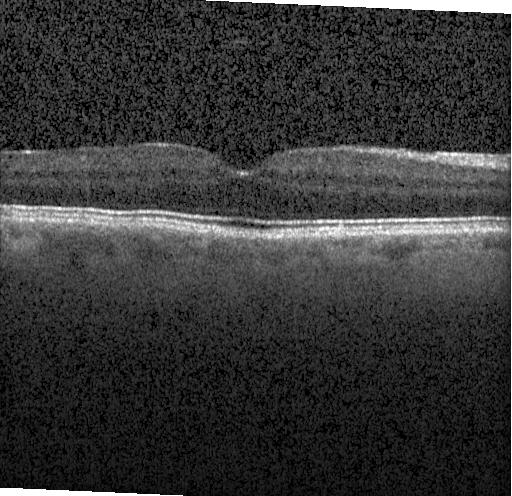

Spectral-domain OCT B-scan: no evidence of choroidal neovascularization, diabetic macular edema, or drusen.